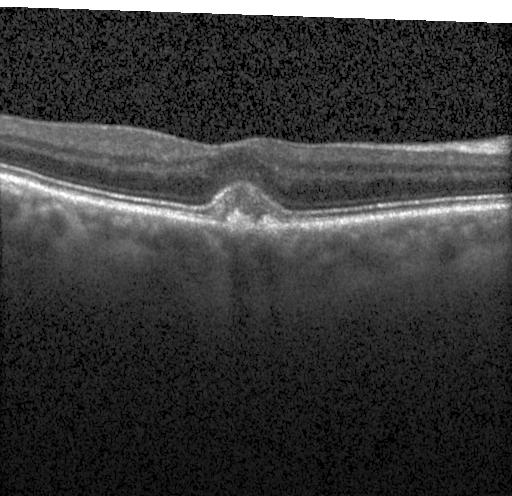 Acquired on a Heidelberg Spectralis; SD-OCT; retinal OCT cross-section; through the macula. Impression: a choroidal neovascular membrane.